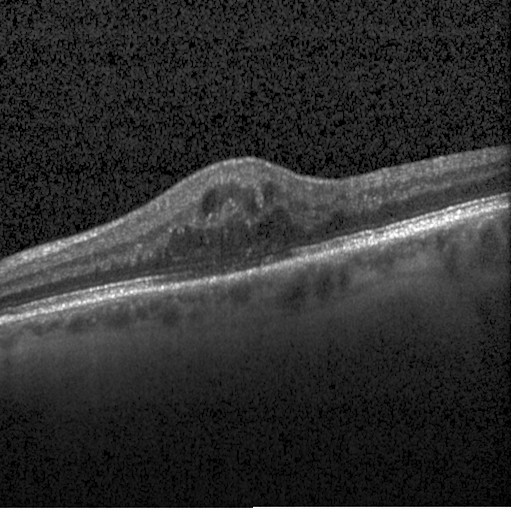
Macular OCT: diabetic macular edema.